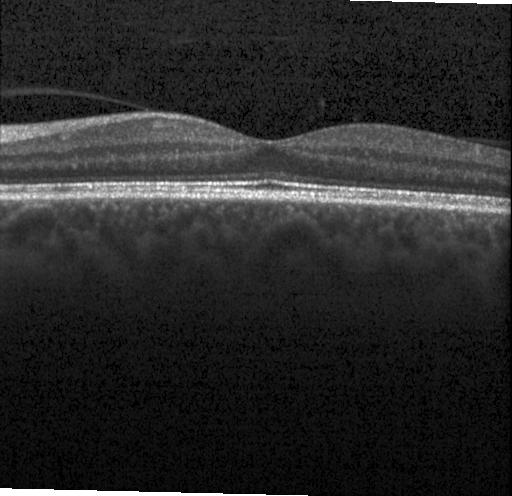
Spectral-domain OCT. OCT B-scan.
Impression: no evidence of choroidal neovascularization, diabetic macular edema, or drusen.